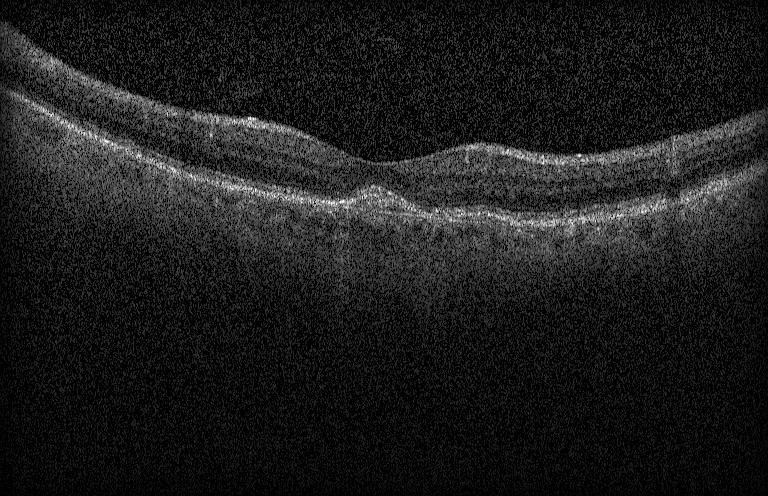 Impression: a choroidal neovascular membrane.